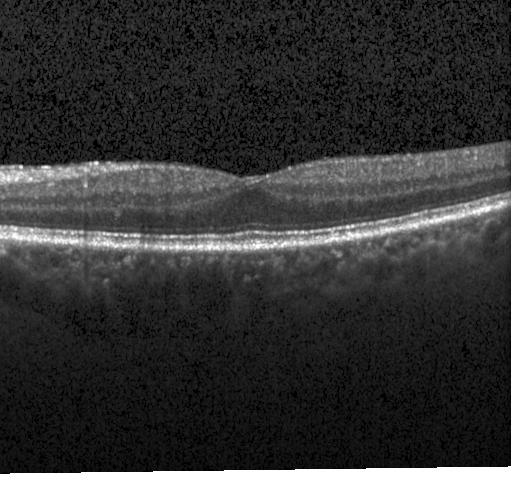
OCT B-scan showing no evidence of choroidal neovascularization, diabetic macular edema, or drusen.